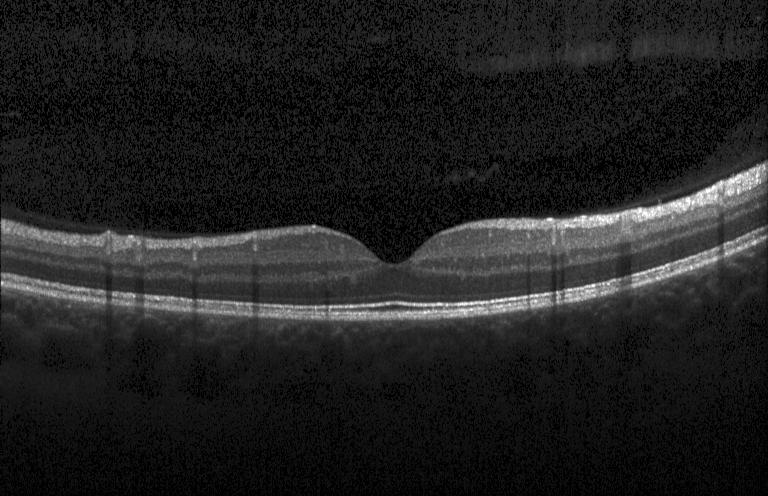

Acquired on a Heidelberg Spectralis, OCT B-scan, spectral-domain OCT.
Dx: no evidence of choroidal neovascularization, diabetic macular edema, or drusen.